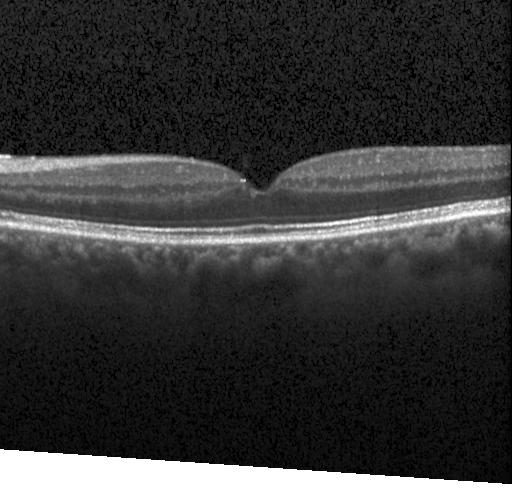
Retinal OCT cross-section — The scan shows no evidence of CNV, DME, or drusen.